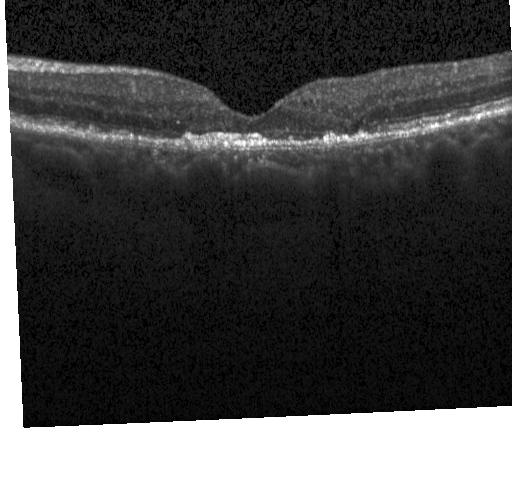
Optical coherence tomography scan · macular scan.
Diagnosis: a choroidal neovascular membrane.